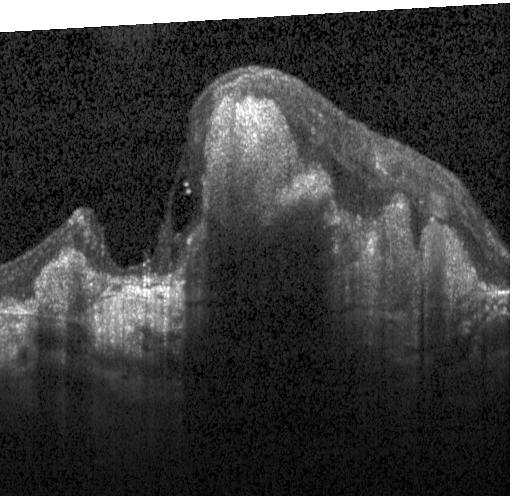
Retinal OCT cross-section, acquired on a Heidelberg Spectralis, macular scan.
The scan shows a choroidal neovascular membrane.